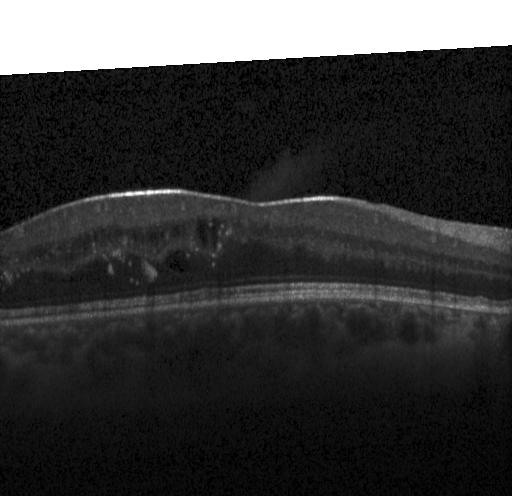
Impression: DME.